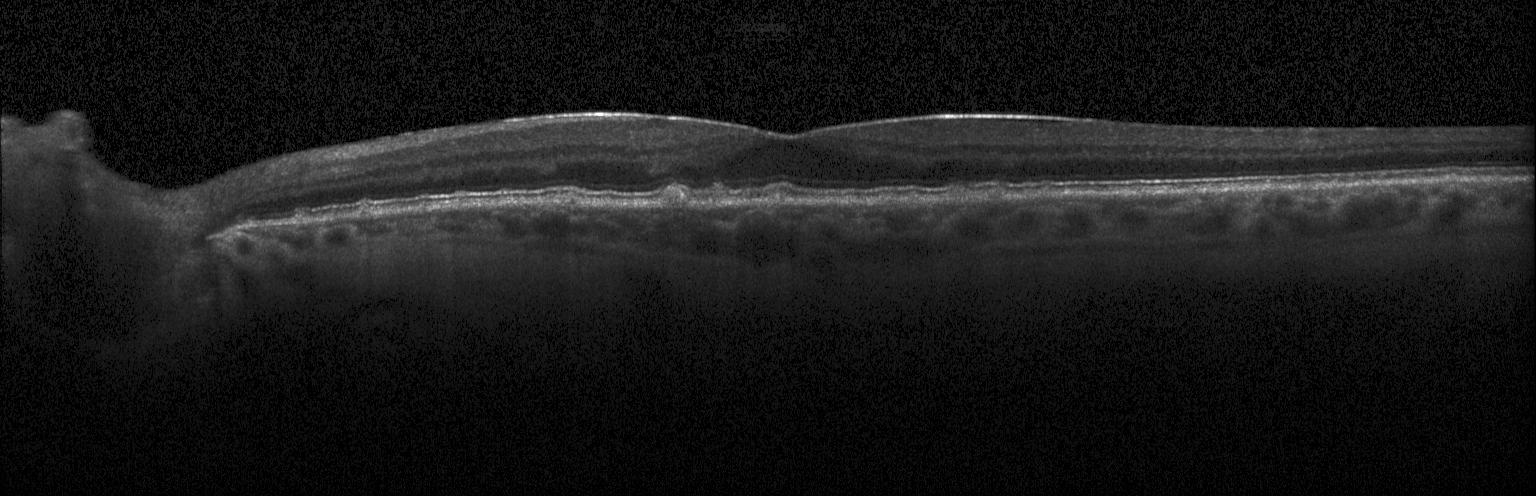 Horizontal scan through the fovea; Heidelberg Spectralis OCT system; retinal OCT B-scan; spectral-domain optical coherence tomography — The scan shows sub-RPE drusenoid deposits.